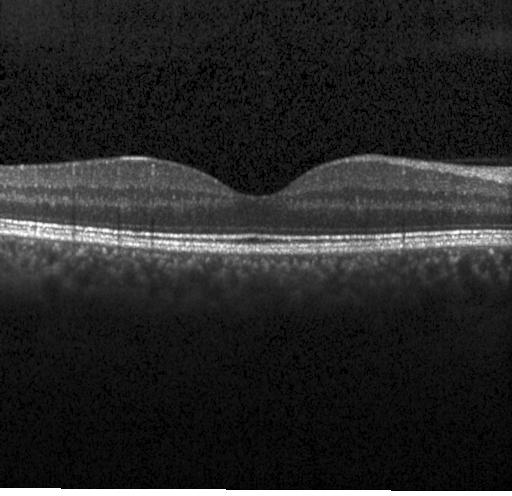
Diagnosis: no evidence of choroidal neovascularization, diabetic macular edema, or drusen.